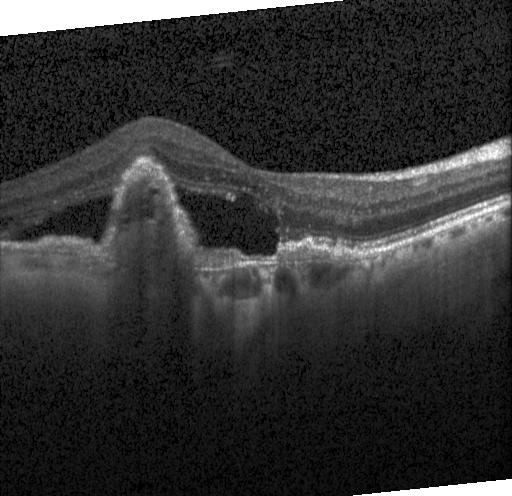 Spectral-domain optical coherence tomography. Centered on the fovea. Instrument: Heidelberg Spectralis. Retinal OCT cross-section — Impression: a choroidal neovascular membrane.